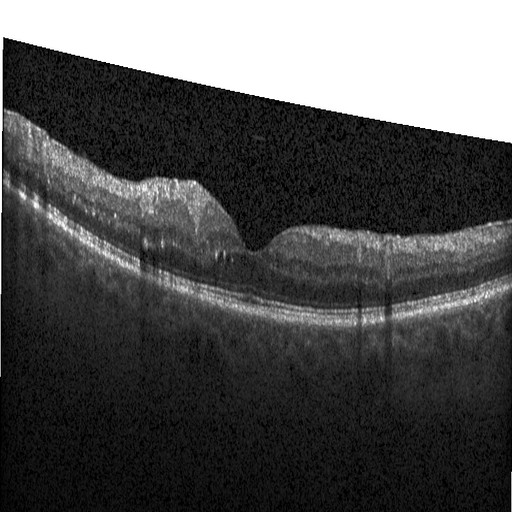
Retinal OCT B-scan · instrument: Heidelberg Spectralis · spectral-domain OCT
Finding: diabetic macular edema.